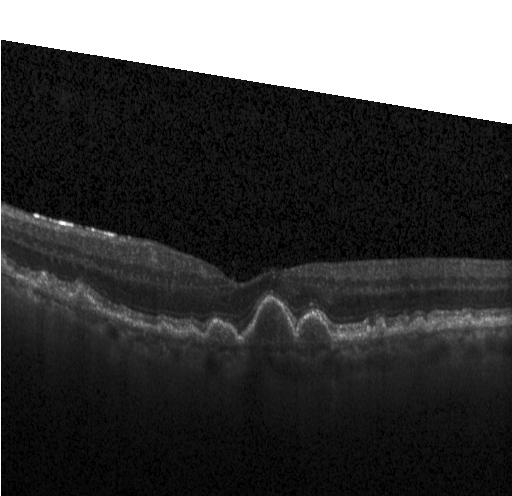 Impression: multiple drusen.